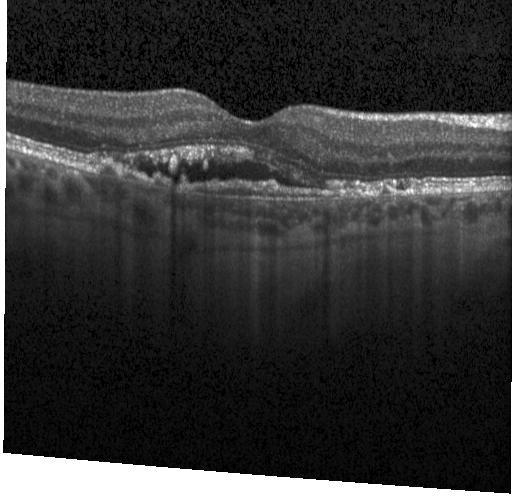 OCT B-scan — Assessment: CNV.